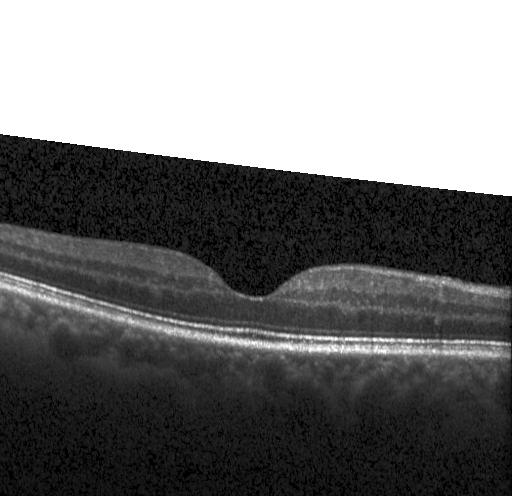
This B-scan demonstrates no CNV, DME, or drusen.